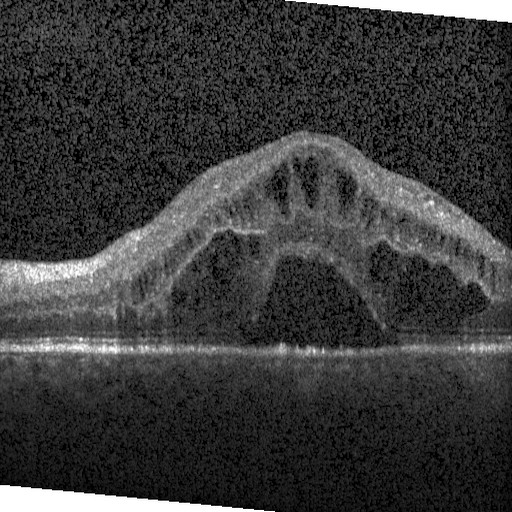
Horizontal scan through the fovea. OCT line scan. Acquired on a Heidelberg Spectralis. Finding: DME.